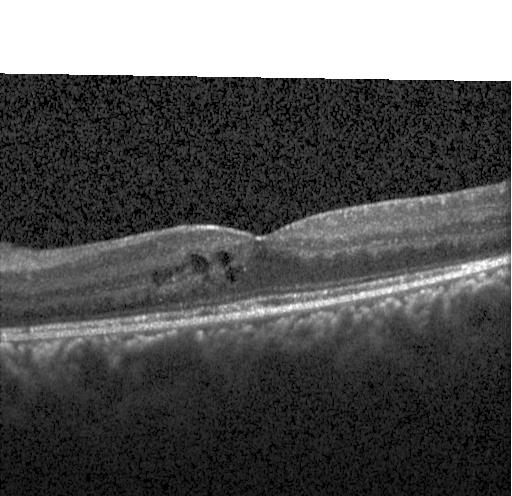
Diagnosis: diabetic macular edema.